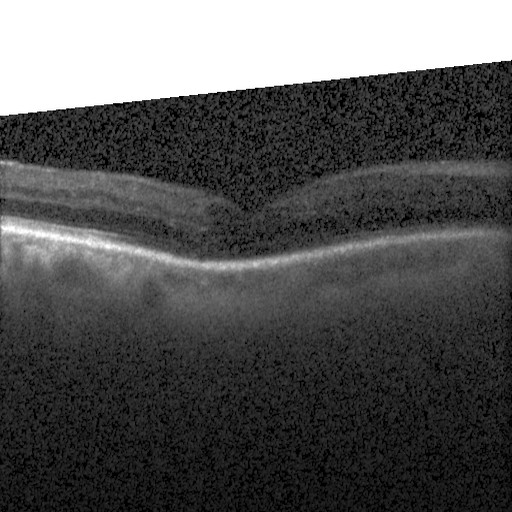
OCT line scan. OCT finding: DME.